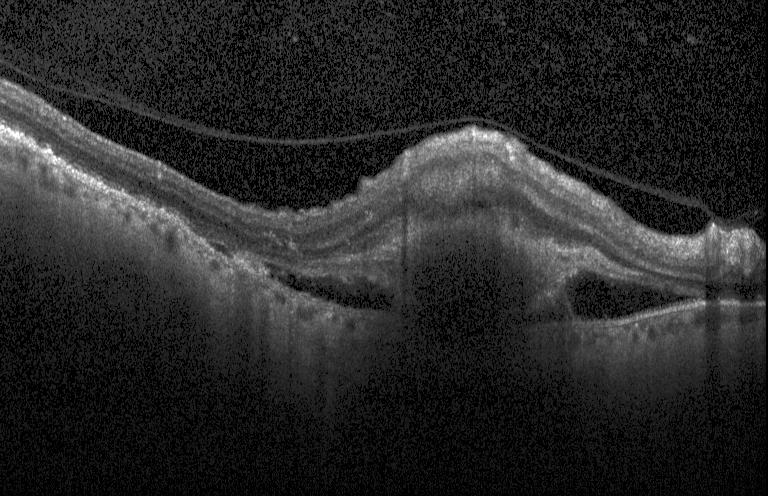
OCT B-scan showing CNV.